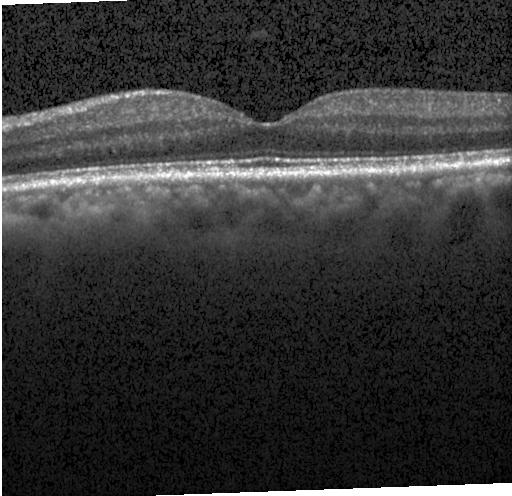

Macular scan · spectral-domain optical coherence tomography · retinal OCT B-scan — Dx: neither CNV, DME, nor drusen.